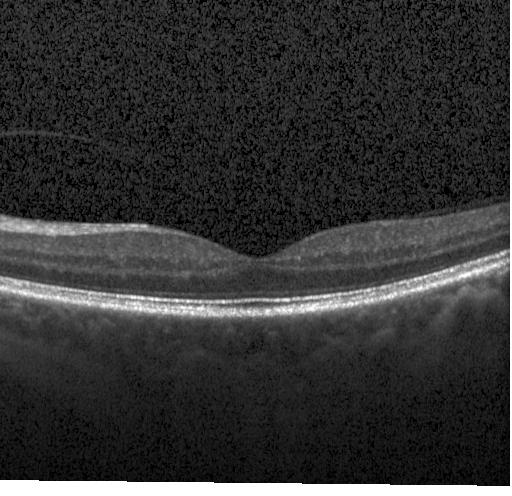 OCT B-scan, horizontal scan through the fovea
Assessment: no evidence of choroidal neovascularization, diabetic macular edema, or drusen.